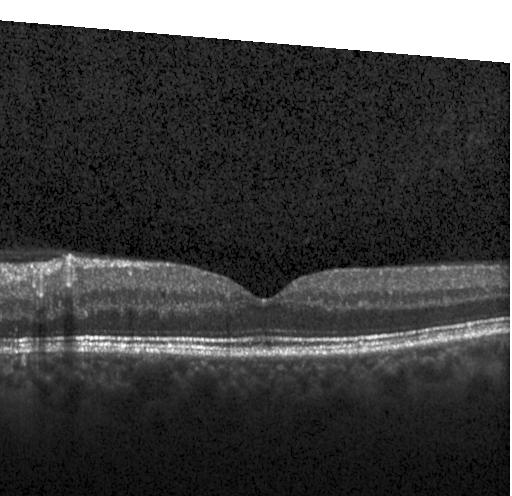 Optical coherence tomography B-scan. The scan shows no choroidal neovascularization, no diabetic macular edema, and no drusen.